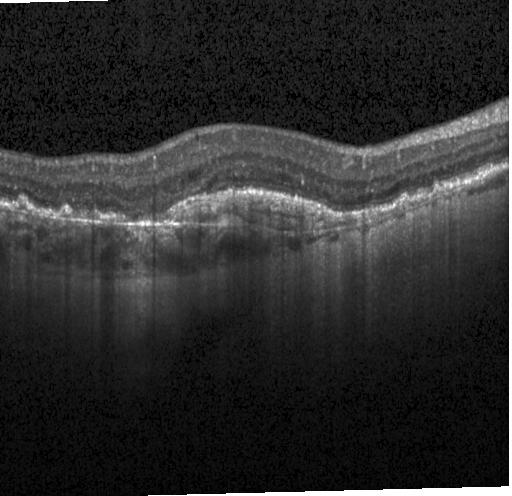 Macular OCT: choroidal neovascularization.